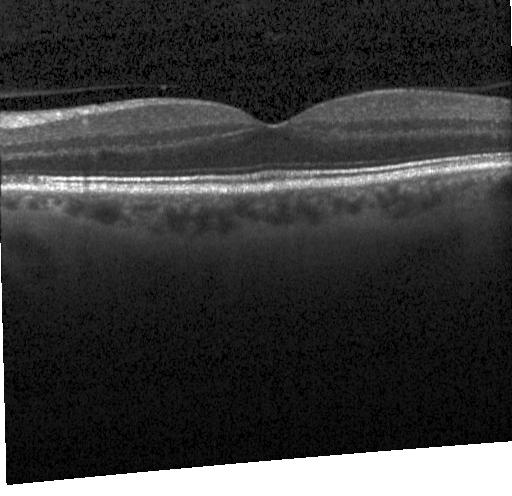 Fovea-centered · acquired on a Heidelberg Spectralis · SD-OCT · retinal OCT cross-section.
Diagnosis: no choroidal neovascularization, no diabetic macular edema, and no drusen.